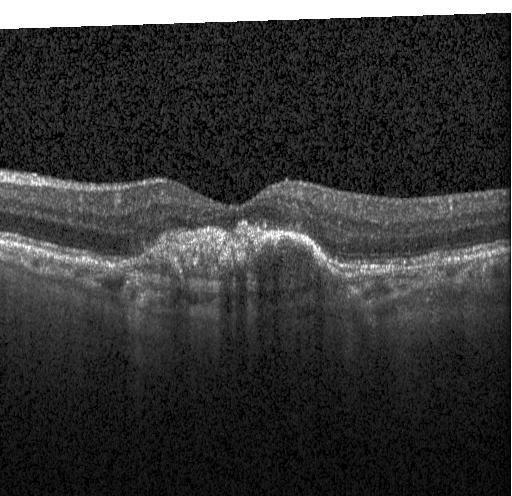

Retinal OCT B-scan.
This B-scan demonstrates choroidal neovascularization.